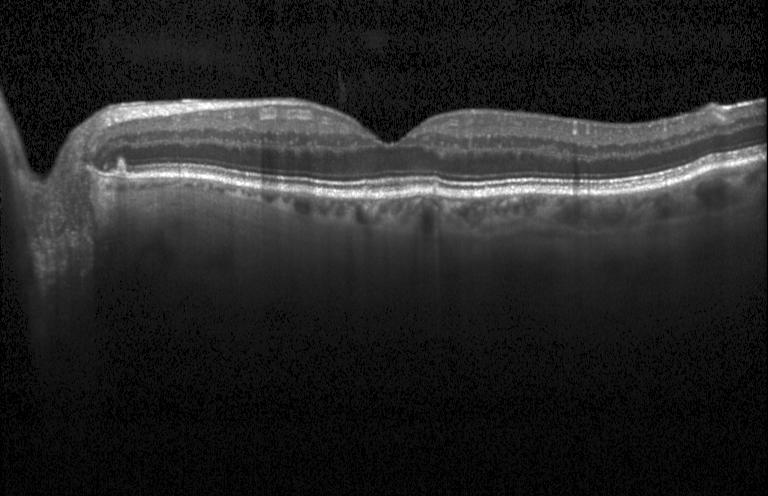
Impression: no evidence of choroidal neovascularization, diabetic macular edema, or drusen.